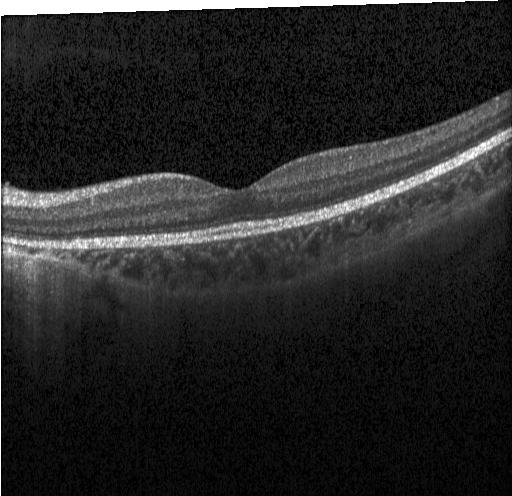
No CNV, no DME, and no drusen.